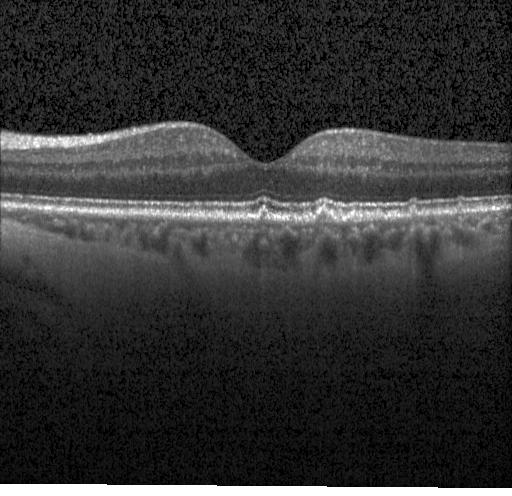 OCT line scan. Sub-RPE drusenoid deposits.